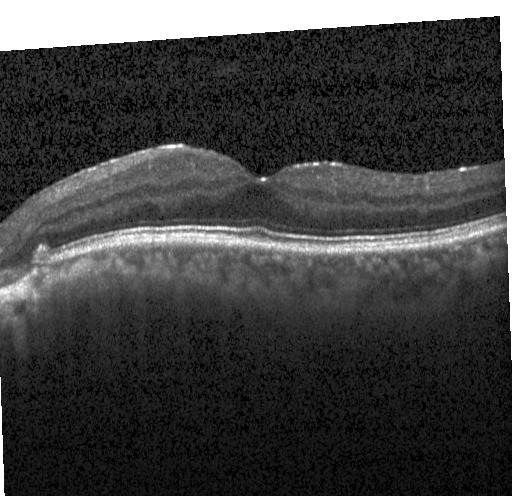
OCT finding: multiple drusen.